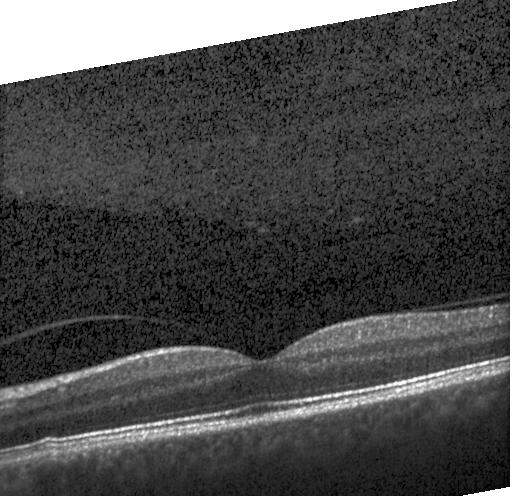
Diagnosis: no CNV, DME, or drusen.